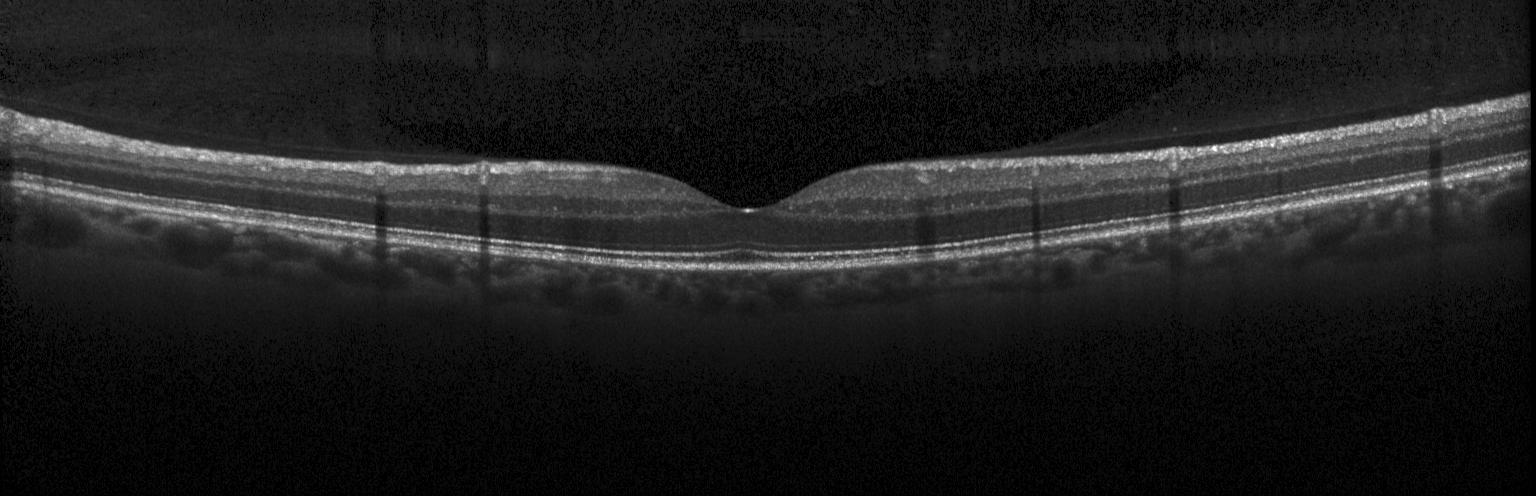 OCT scan showing no evidence of choroidal neovascularization, diabetic macular edema, or drusen.